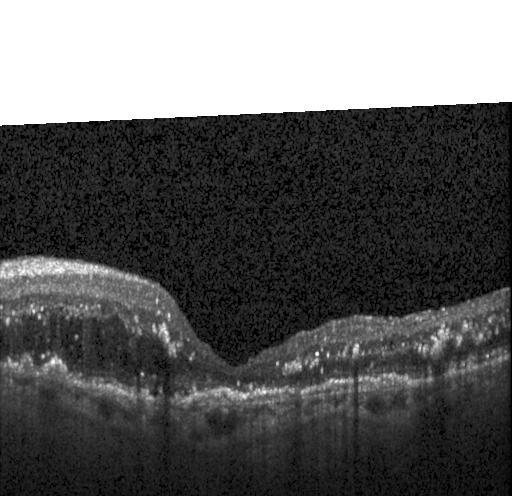

Acquired on a Heidelberg Spectralis. Retinal OCT cross-section. This B-scan demonstrates choroidal neovascularization (CNV).